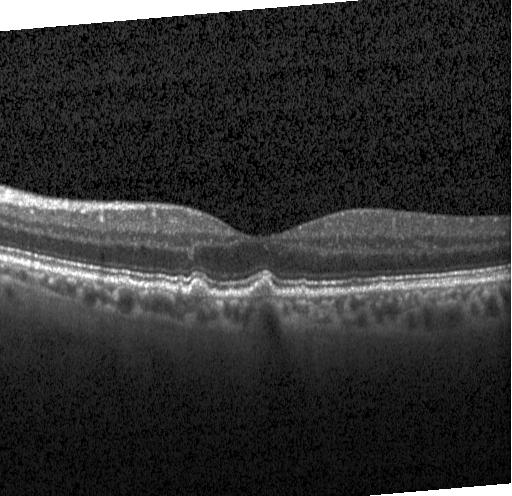 OCT line scan
OCT finding: drusen.